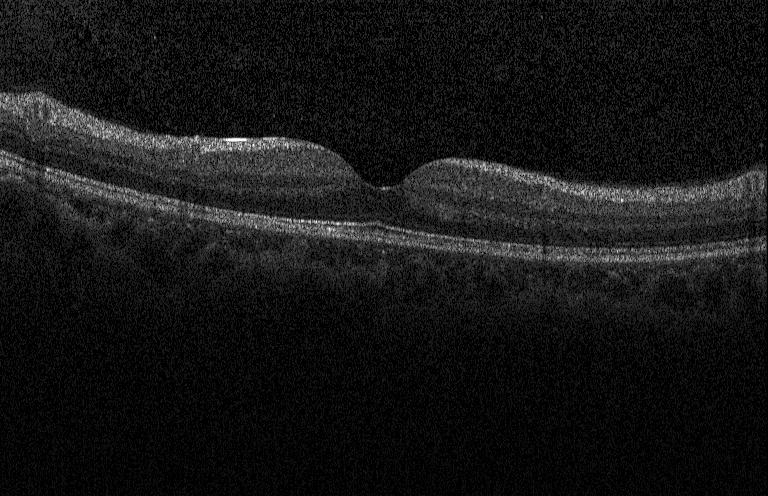 Impression: neither choroidal neovascularization, diabetic macular edema, nor drusen.